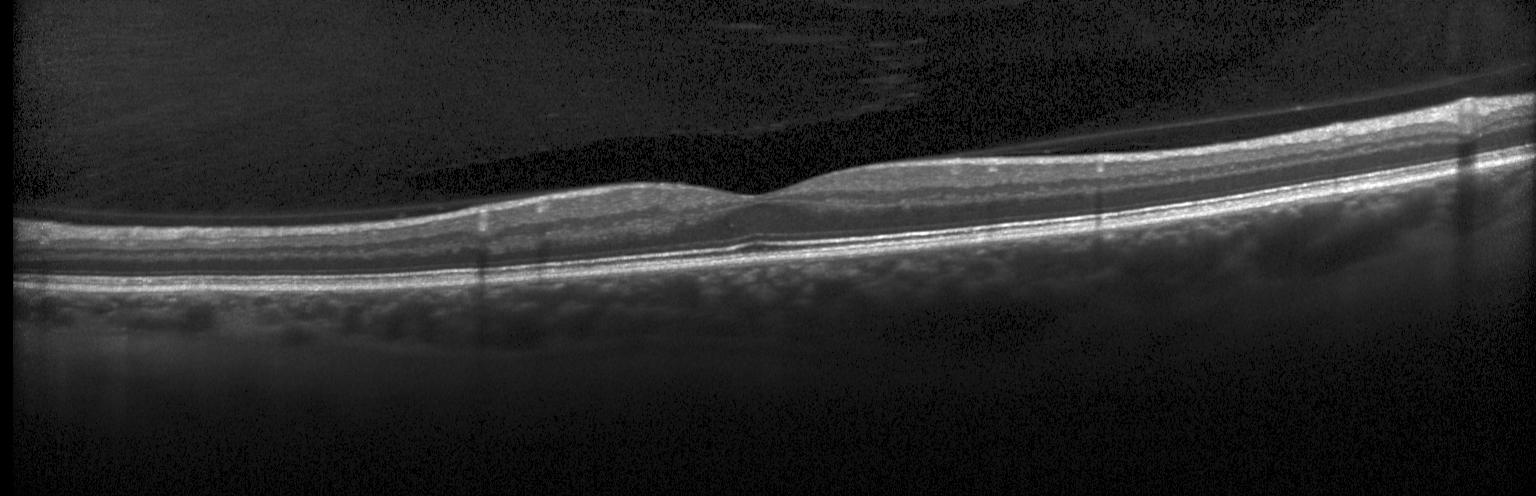 OCT B-scan; SD-OCT; instrument: Heidelberg Spectralis. OCT finding: neither choroidal neovascularization, diabetic macular edema, nor drusen.